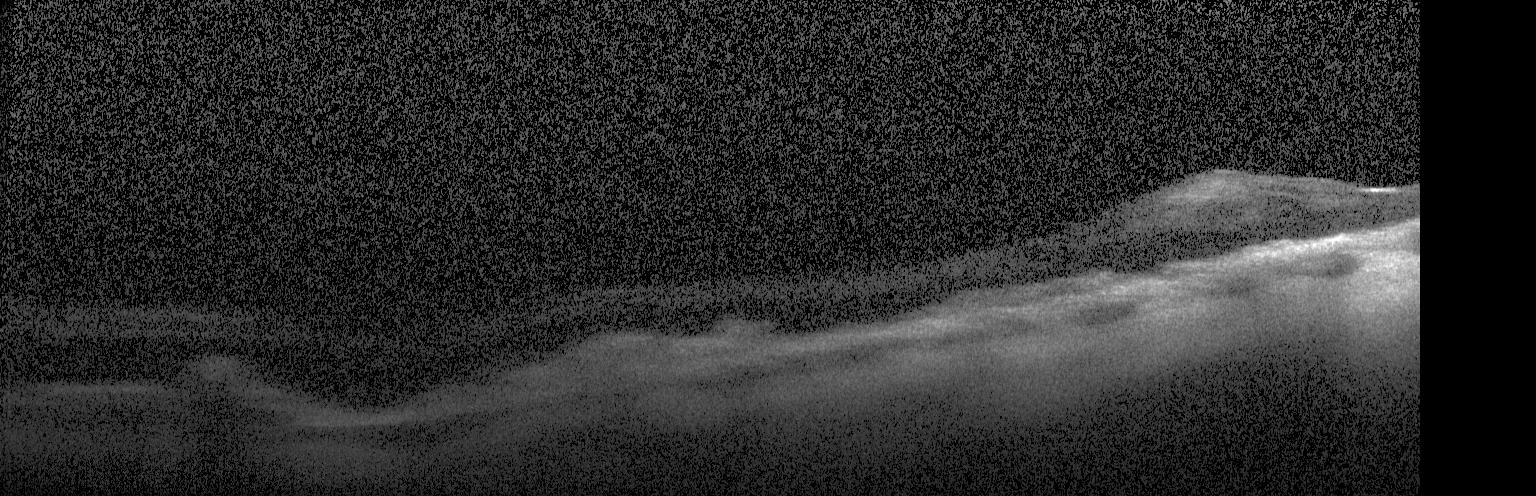 Retinal OCT B-scan
The scan shows choroidal neovascularization (CNV).